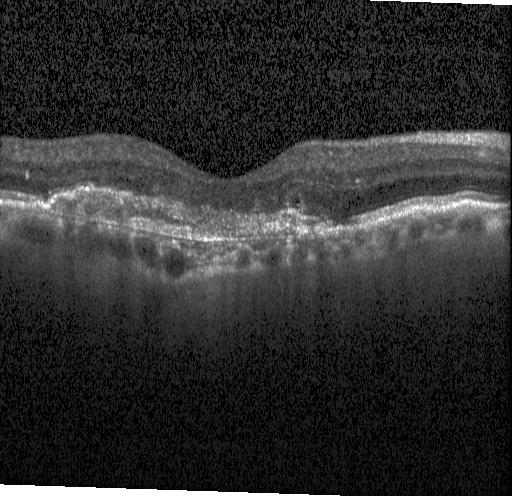 Macular OCT demonstrating a choroidal neovascular membrane.